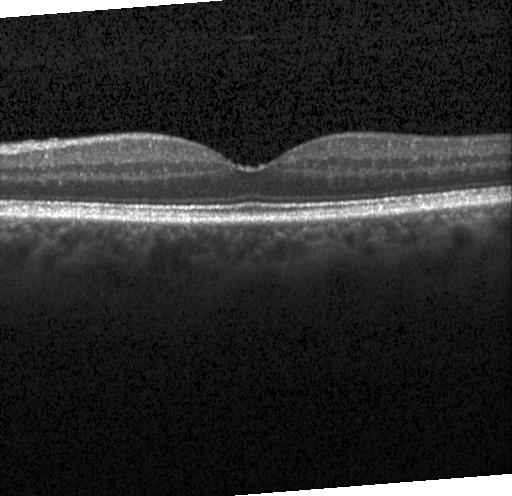

Assessment: neither CNV, DME, nor drusen.